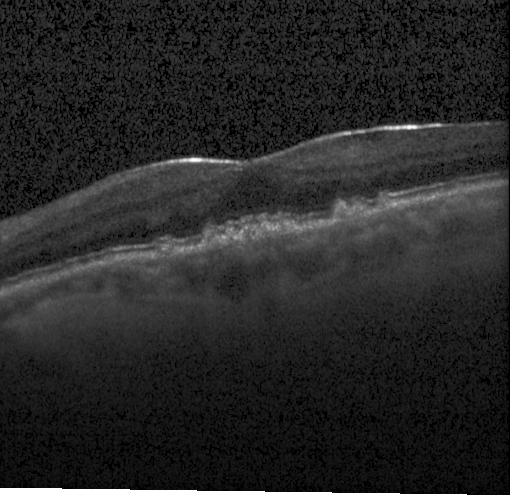
OCT B-scan · spectral-domain optical coherence tomography.
Drusen.